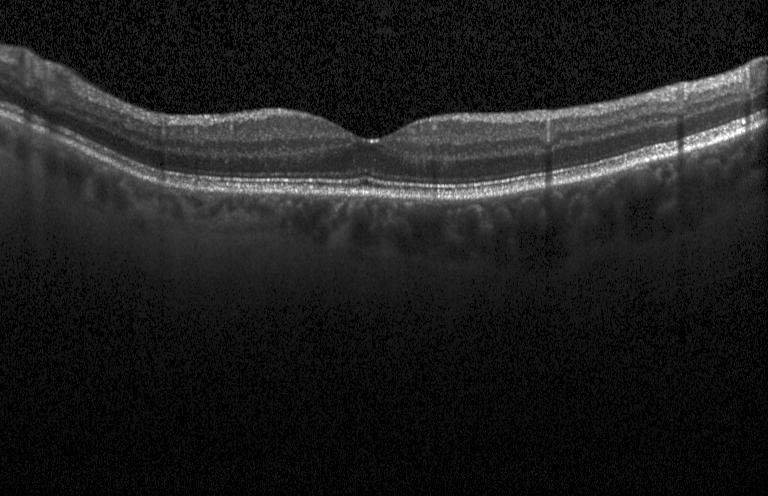

OCT B-scan, spectral-domain optical coherence tomography, horizontal scan through the fovea
Finding: no evidence of choroidal neovascularization, diabetic macular edema, or drusen.